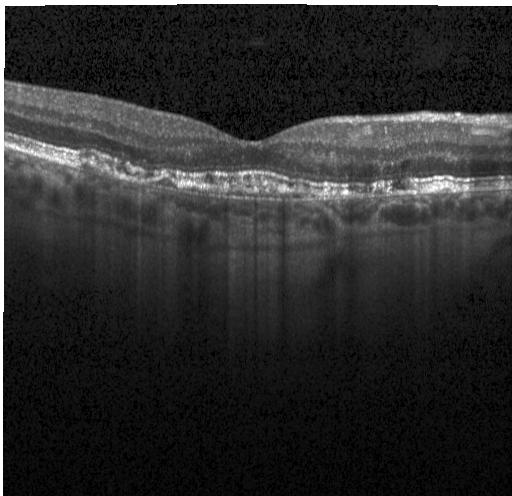 OCT scan showing a choroidal neovascular membrane.